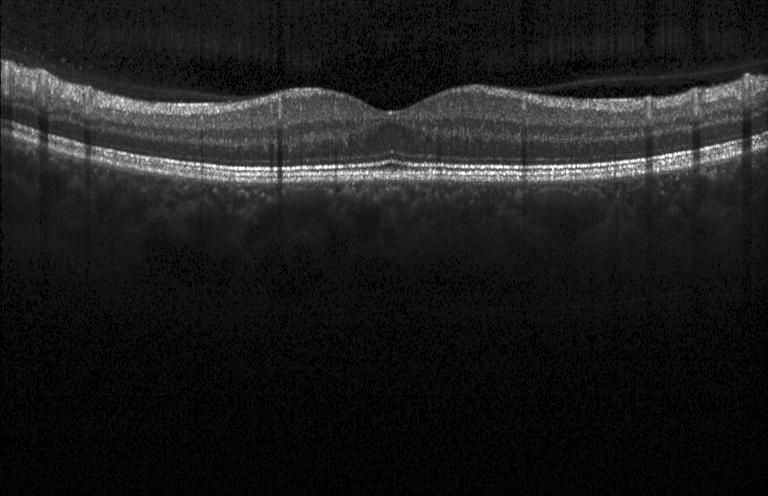
Finding: no CNV, DME, or drusen.